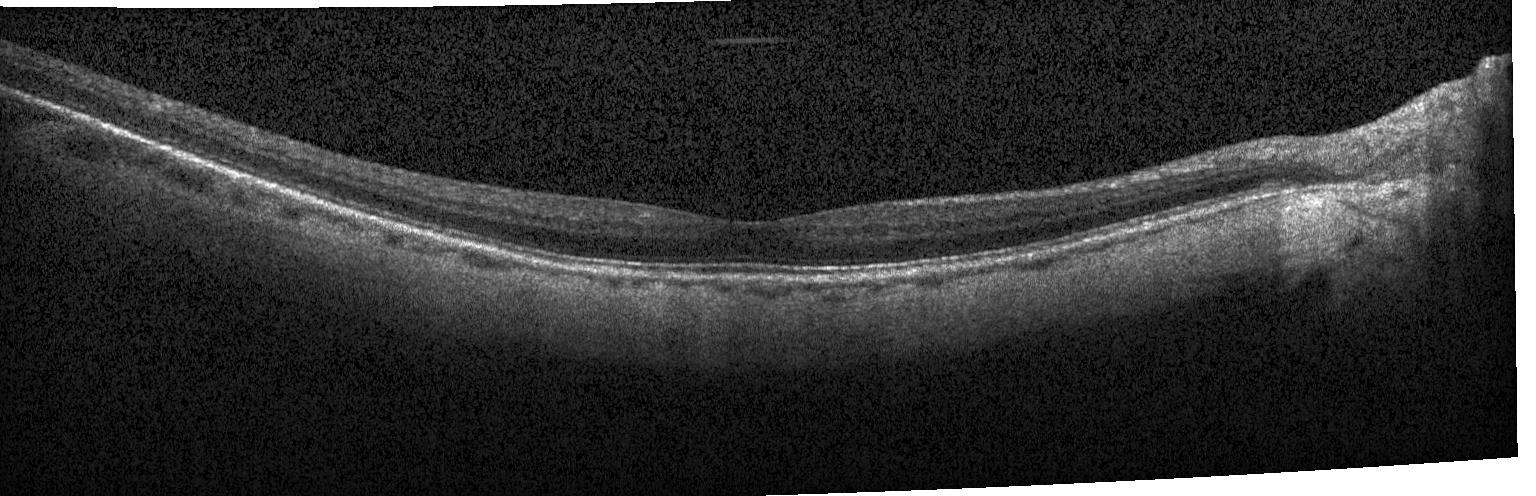

Spectral-domain OCT. Acquired on a Heidelberg Spectralis. Optical coherence tomography B-scan.
Diagnosis: no choroidal neovascularization, diabetic macular edema, or drusen.